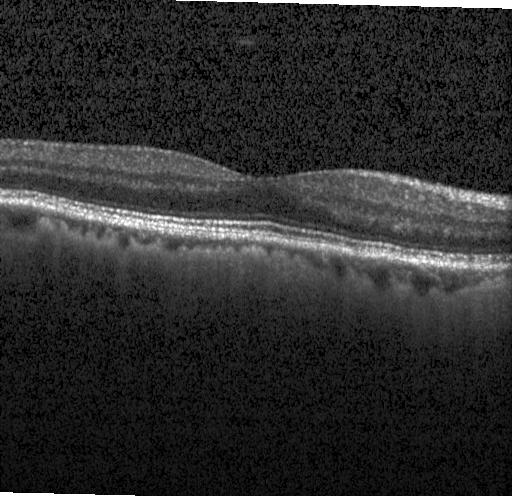 Centered on the fovea · retinal OCT B-scan. Assessment: no CNV, DME, or drusen.